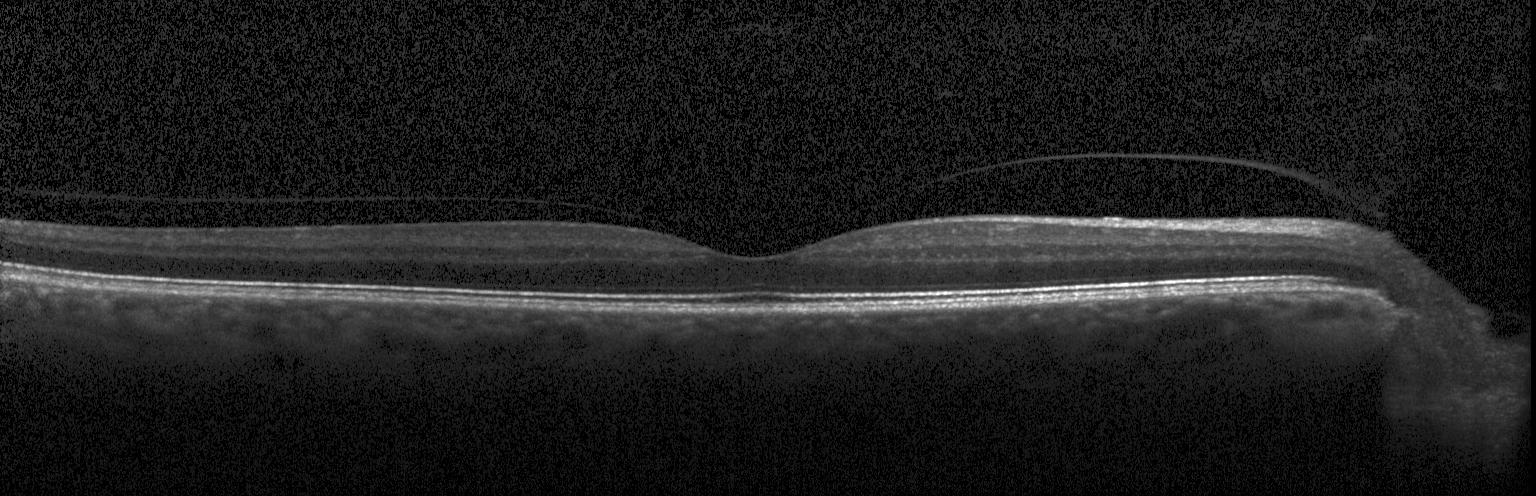 Optical coherence tomography scan · spectral-domain OCT · horizontal scan through the fovea
Diagnosis: no CNV, no DME, and no drusen.